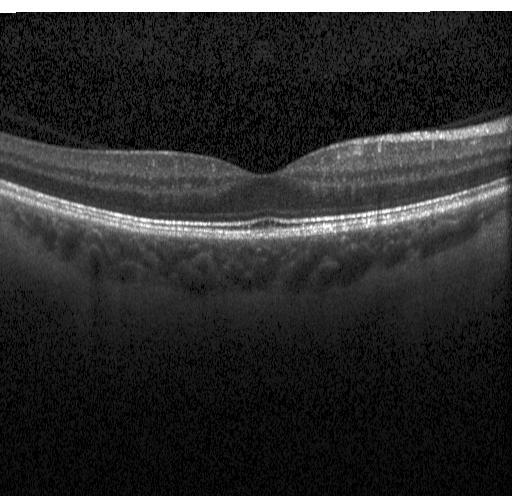 Dx: no evidence of choroidal neovascularization, diabetic macular edema, or drusen.